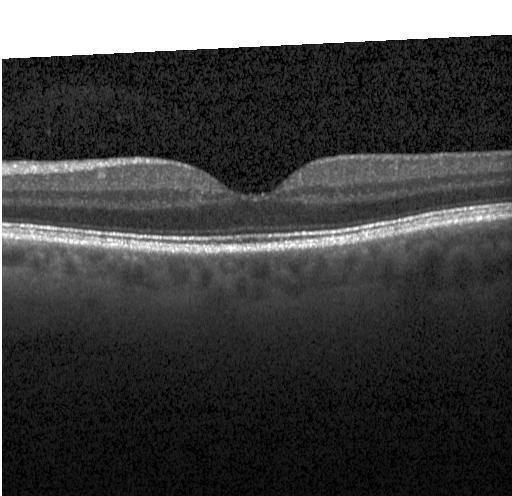
Assessment: no evidence of choroidal neovascularization, diabetic macular edema, or drusen.